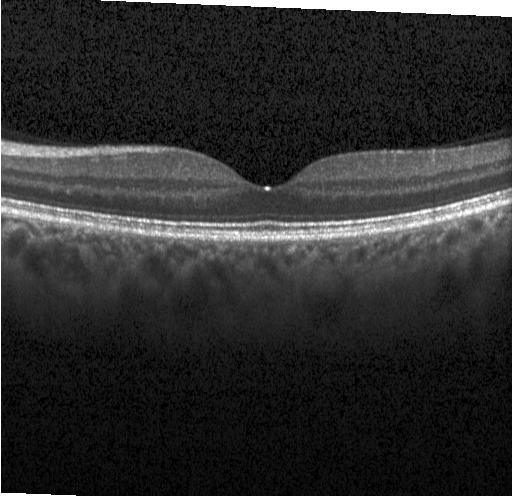
This B-scan demonstrates no choroidal neovascularization, diabetic macular edema, or drusen.